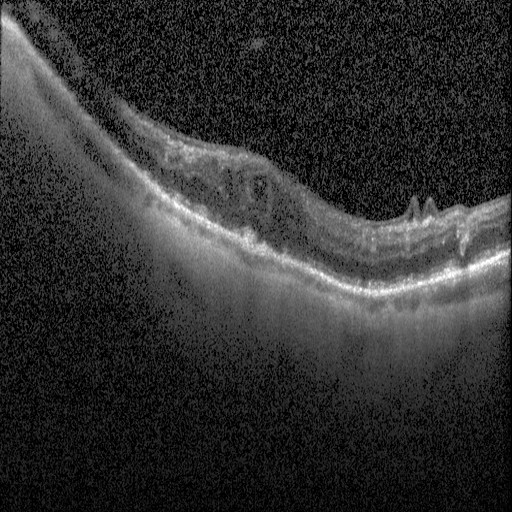 Spectral-domain OCT B-scan: diabetic macular edema.